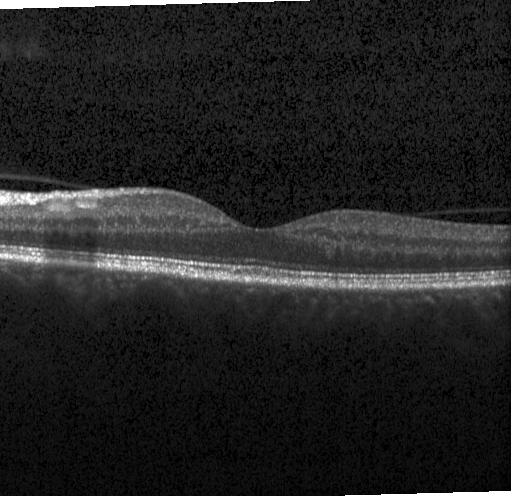 Macular OCT: no CNV, DME, or drusen.